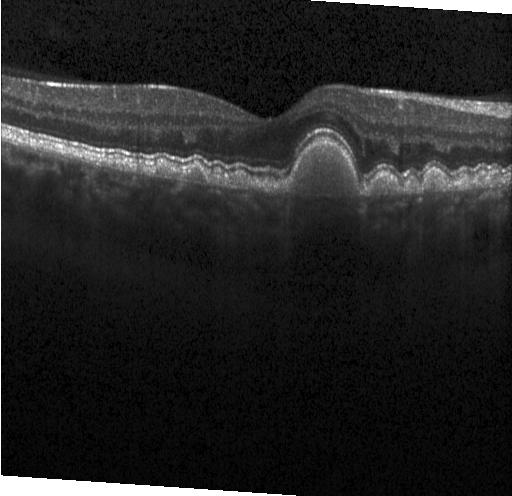
Retinal OCT cross-section showing drusen.